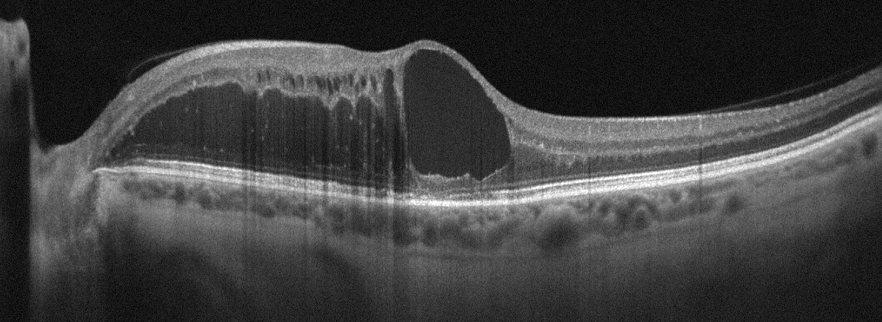 Fovea-centered, acquired on an Optovue Avanti RTVue XR, optical coherence tomography scan
Macular OCT: retinal vein occlusion (RVO).